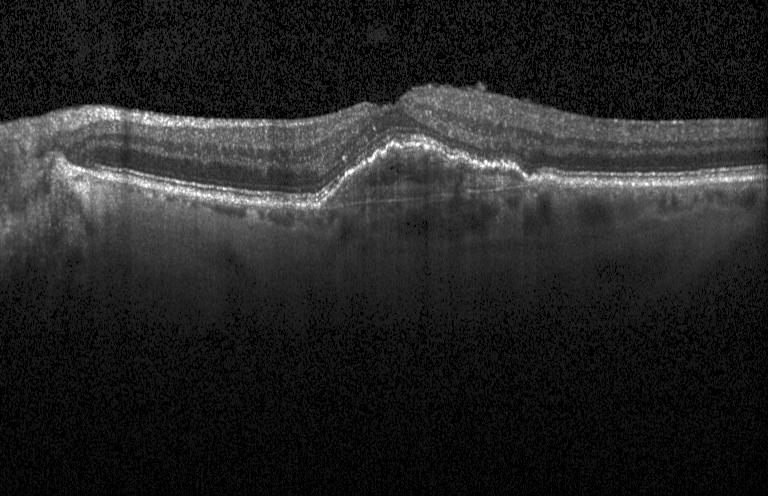
Spectral-domain optical coherence tomography · OCT B-scan · centered on the fovea · instrument: Heidelberg Spectralis.
Diagnosis: choroidal neovascularization (CNV).